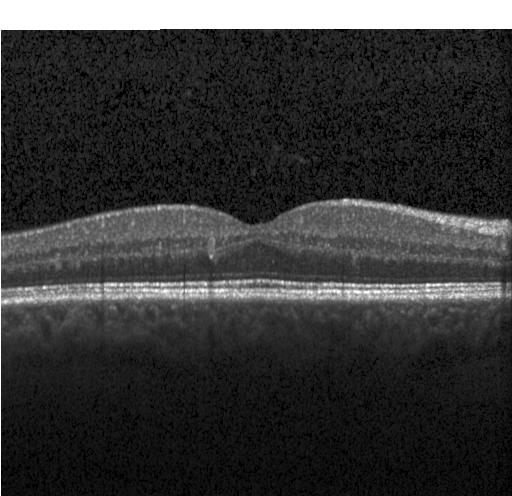
Acquired on a Heidelberg Spectralis · OCT line scan.
Assessment: no choroidal neovascularization, diabetic macular edema, or drusen.